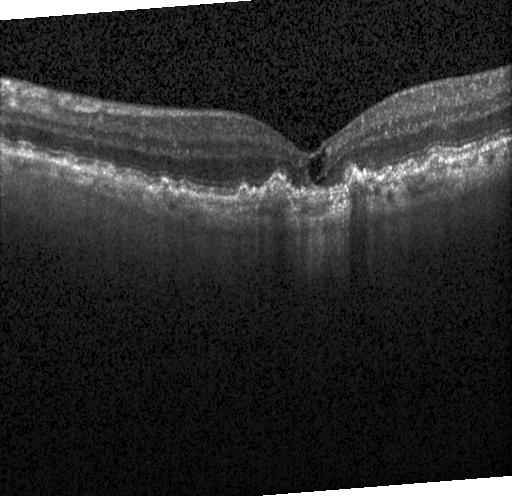
Acquired on a Heidelberg Spectralis. Optical coherence tomography scan. Spectral-domain optical coherence tomography. Centered on the fovea. Diagnosis: choroidal neovascularization (CNV).